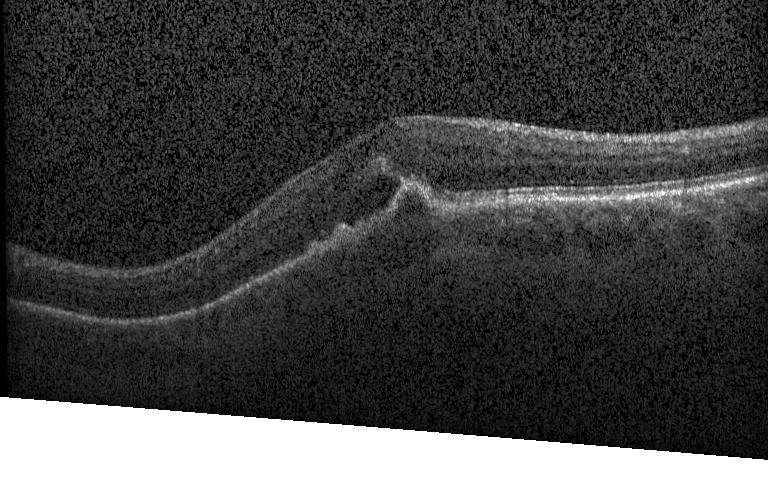

Retinal OCT cross-section.
The scan shows choroidal neovascularization (CNV).